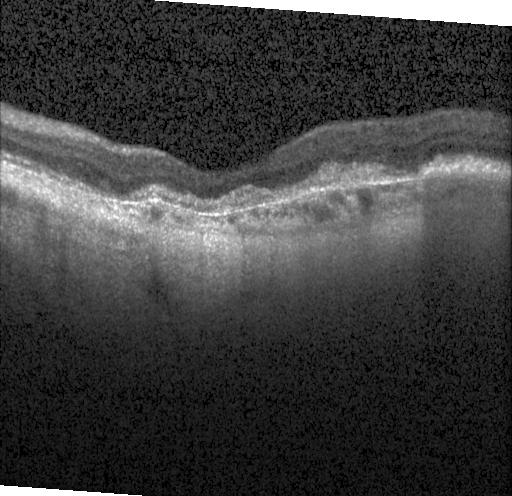 Acquired on a Heidelberg Spectralis, optical coherence tomography B-scan, centered on the fovea, SD-OCT.
Diagnosis: CNV.